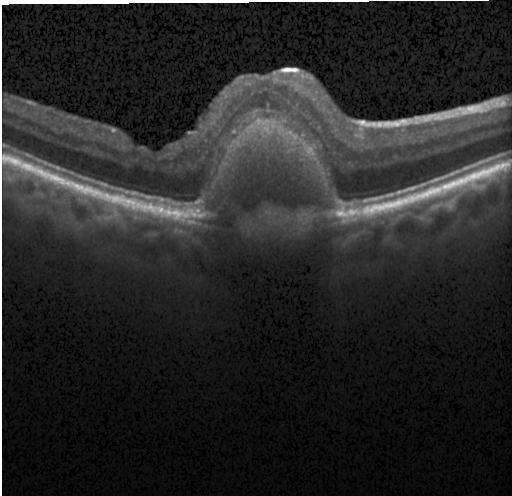

Retinal OCT cross-section, through the macula — Dx: a choroidal neovascular membrane.